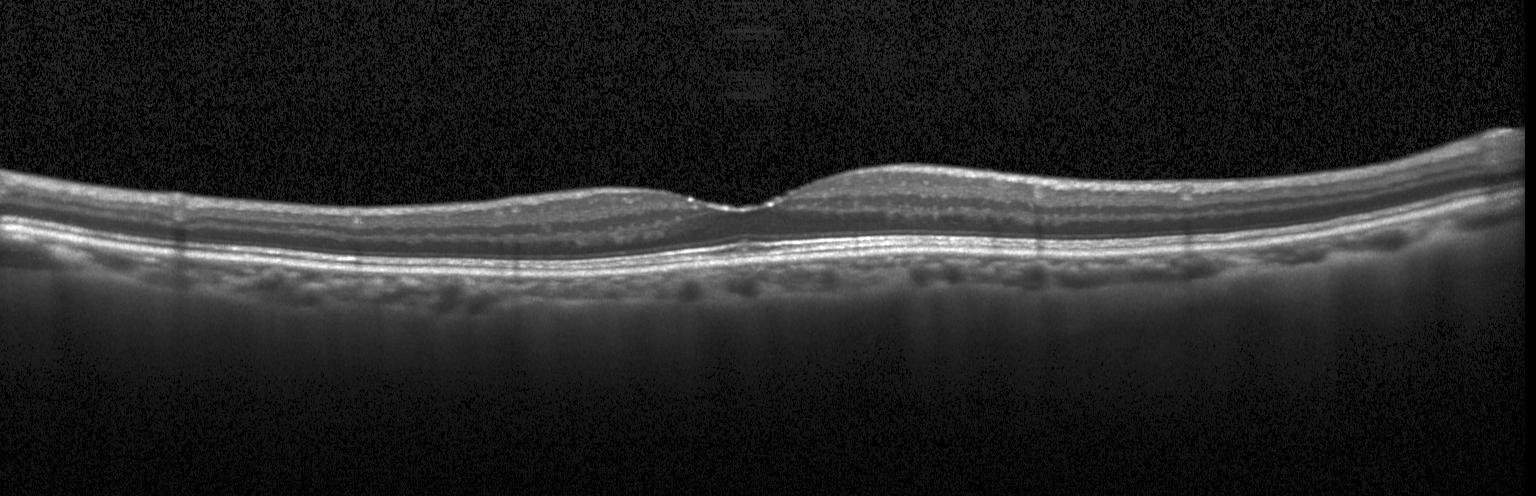
Optical coherence tomography scan. Impression: no evidence of CNV, DME, or drusen.